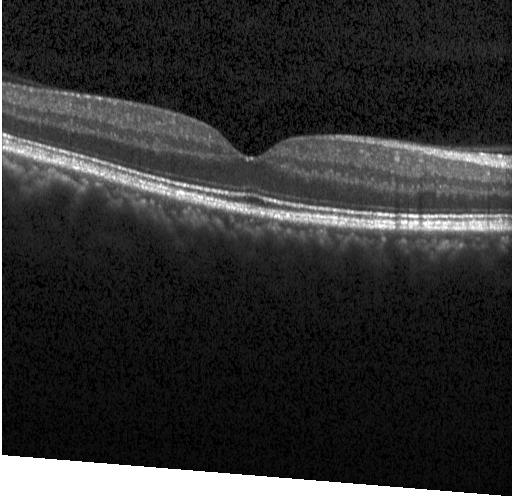
Diagnosis: no choroidal neovascularization, no diabetic macular edema, and no drusen.